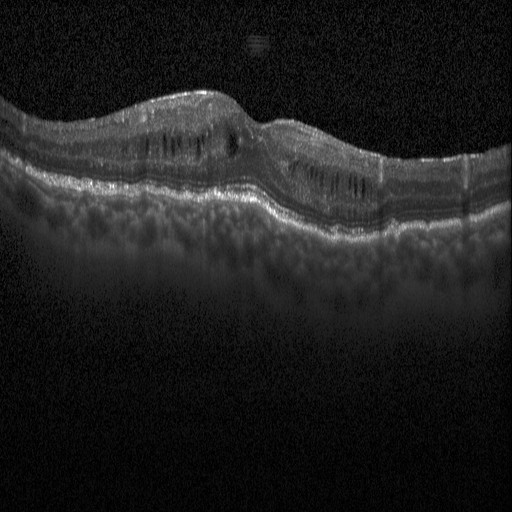 Macular OCT: diabetic macular edema.